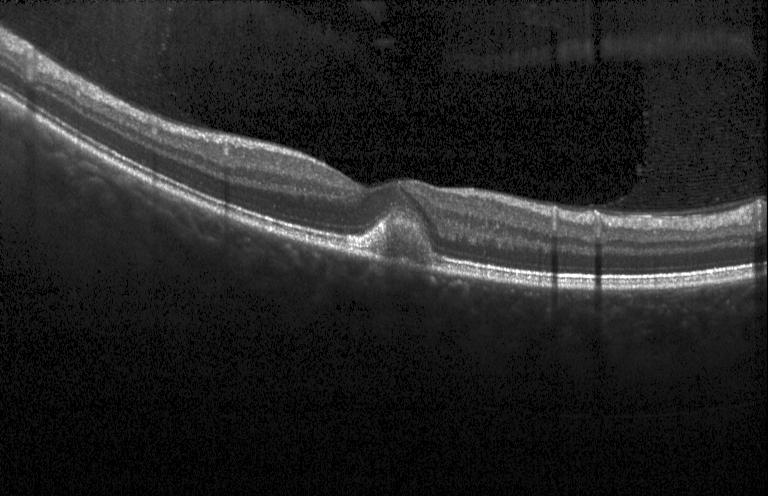
OCT B-scan. This B-scan demonstrates drusen.